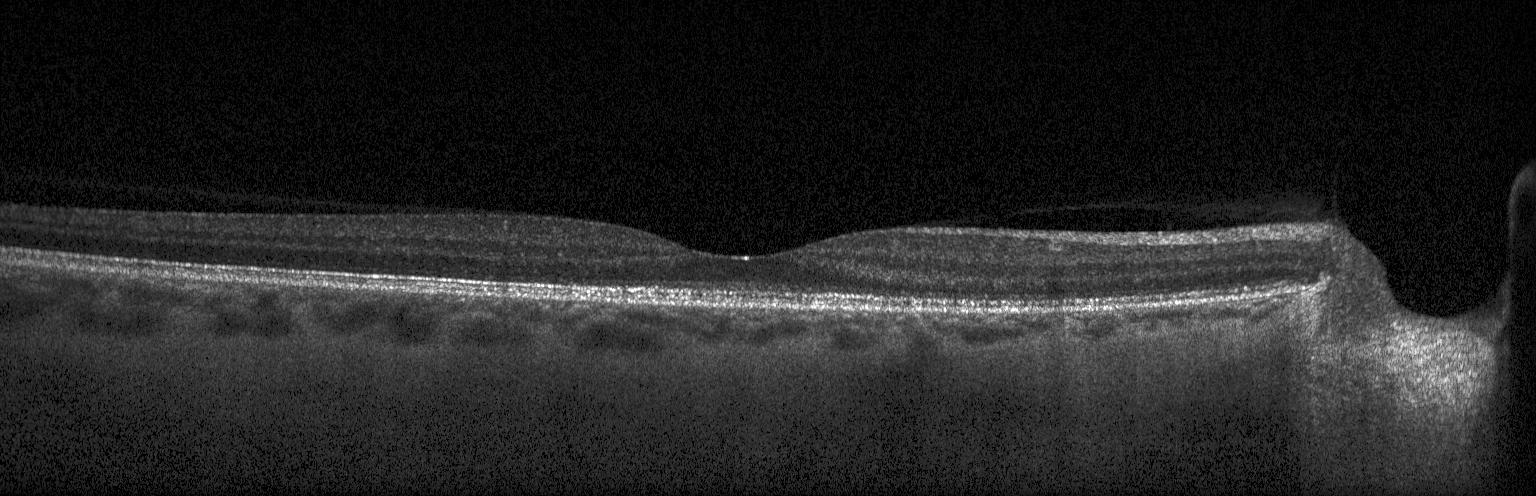

Instrument: Heidelberg Spectralis, spectral-domain OCT, retinal OCT cross-section. Impression: neither choroidal neovascularization, diabetic macular edema, nor drusen.